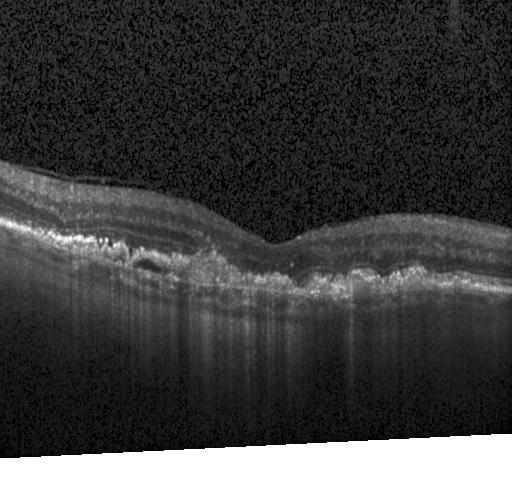

Retinal OCT B-scan
Macular OCT: a choroidal neovascular membrane.